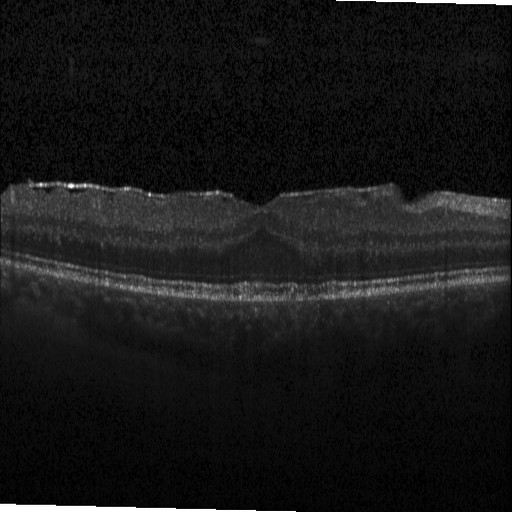
Impression: diabetic macular edema (DME).